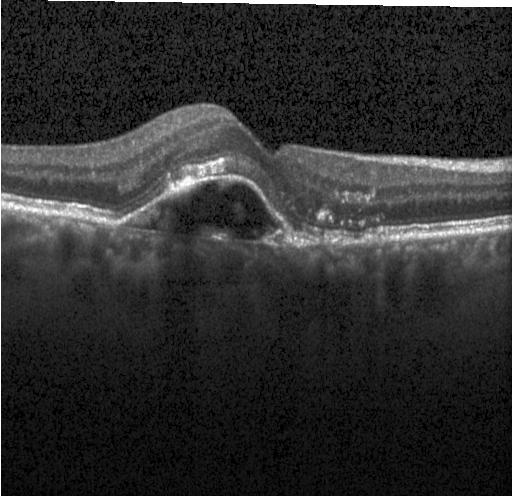 Dx: a choroidal neovascular membrane.